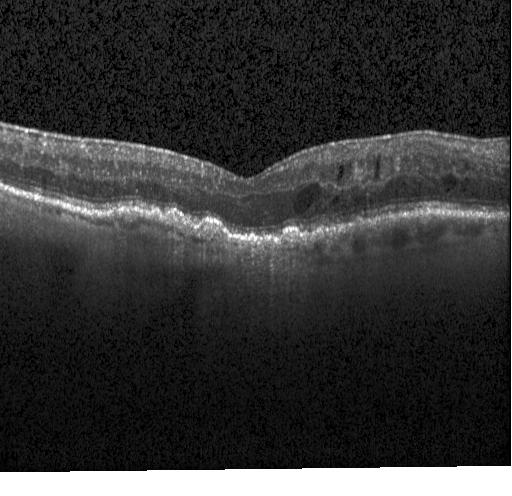
Instrument: Heidelberg Spectralis, OCT B-scan. Impression: a choroidal neovascular membrane.